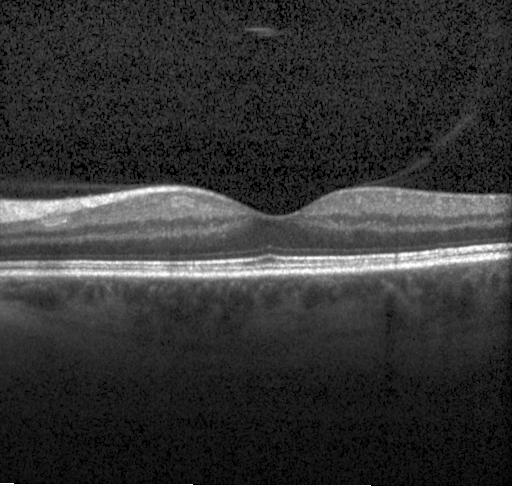 Assessment: no choroidal neovascularization, diabetic macular edema, or drusen.